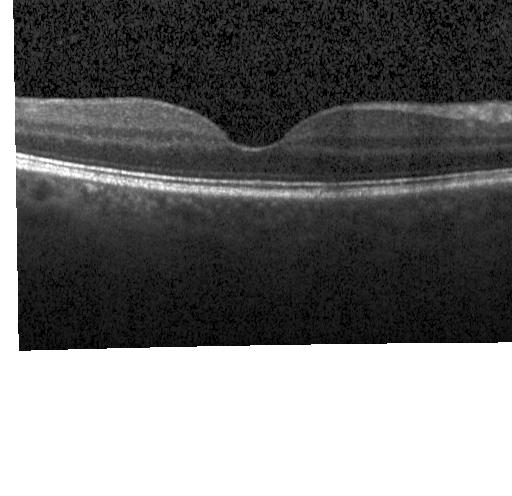
Horizontal scan through the fovea · spectral-domain OCT · Heidelberg Spectralis OCT system · retinal OCT B-scan.
Assessment: no evidence of CNV, DME, or drusen.